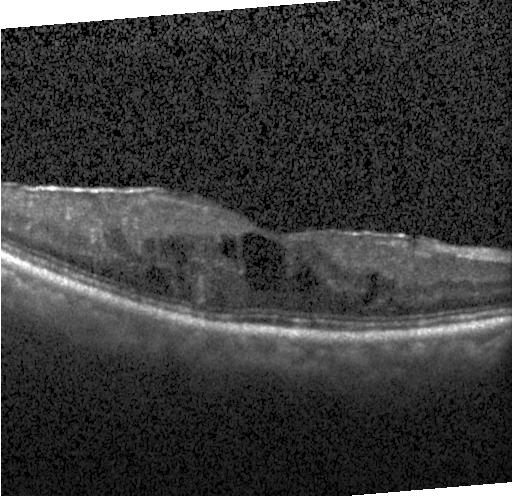

Spectral-domain optical coherence tomography. Instrument: Heidelberg Spectralis. Centered on the fovea. OCT line scan.
This B-scan demonstrates diabetic macular edema (DME).